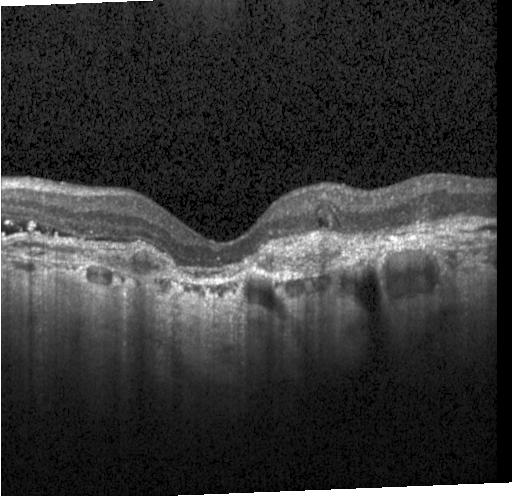 Optical coherence tomography B-scan — Impression: a choroidal neovascular membrane.